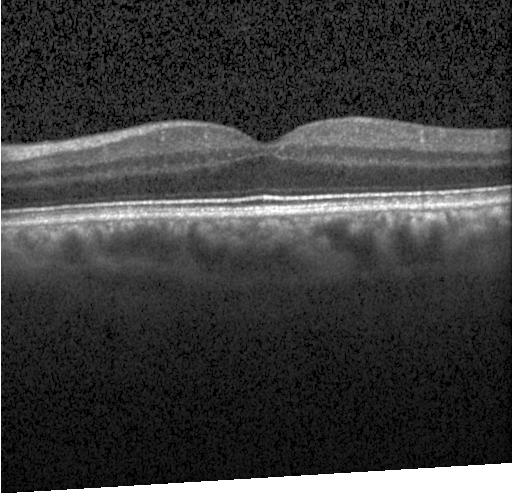
Spectral-domain OCT B-scan: no CNV, no DME, and no drusen.